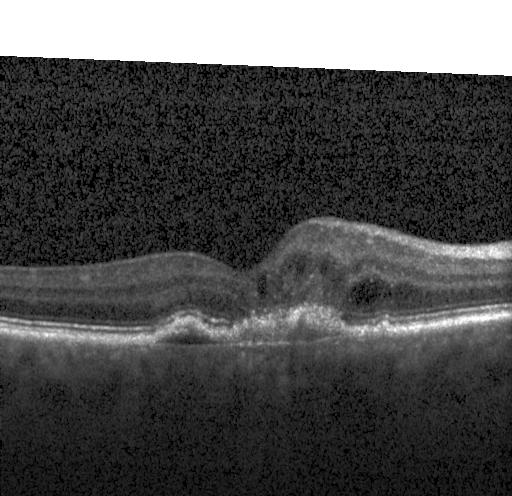
OCT B-scan showing choroidal neovascularization.